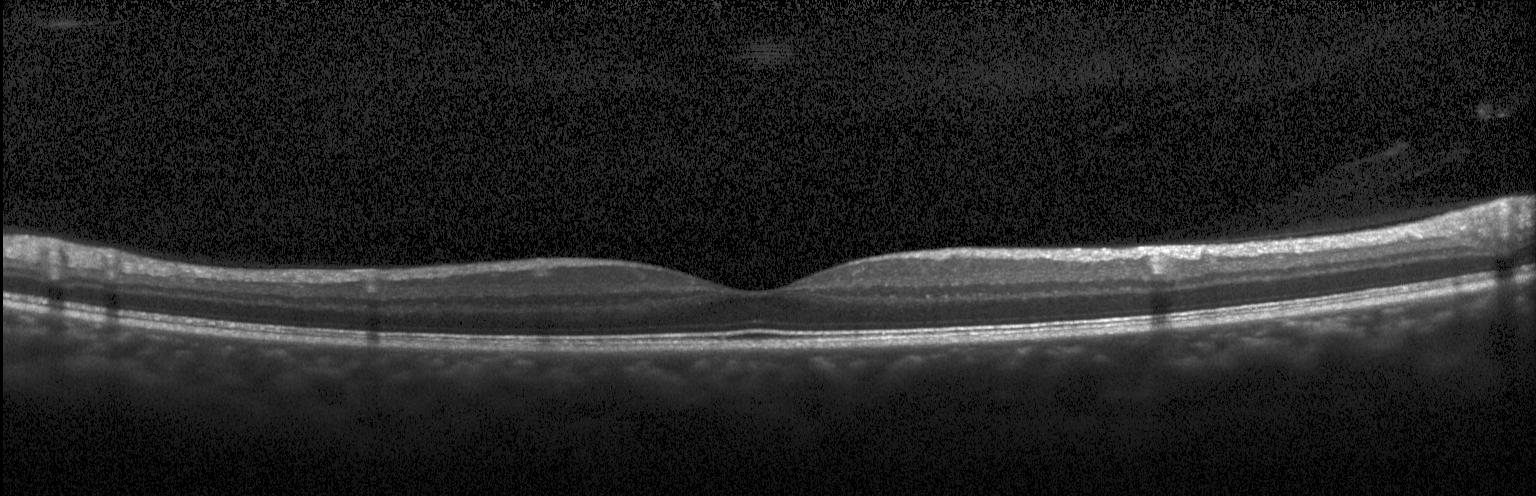 Diagnosis: no CNV, DME, or drusen.